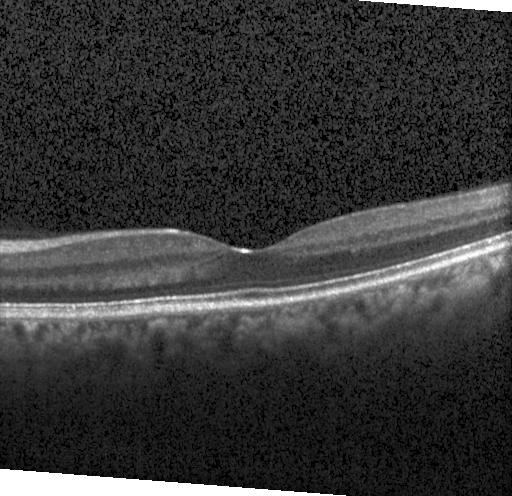

Dx: no evidence of choroidal neovascularization, diabetic macular edema, or drusen.